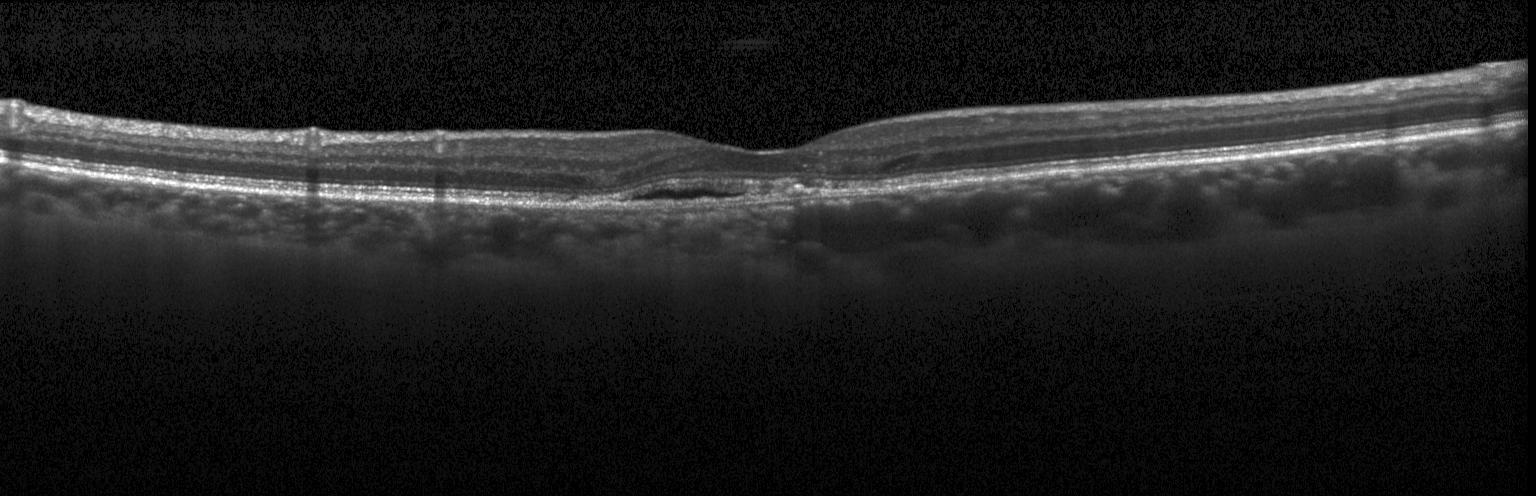
Acquired on a Heidelberg Spectralis. Spectral-domain optical coherence tomography. Optical coherence tomography scan. OCT finding: choroidal neovascularization.